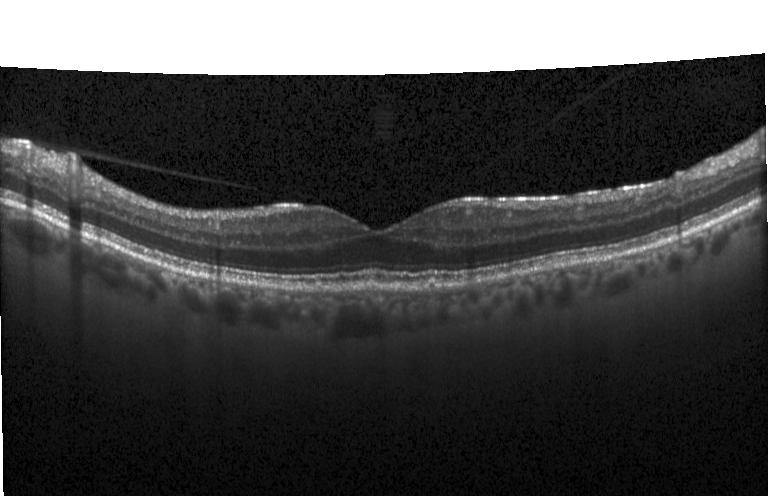

Spectral-domain optical coherence tomography; Heidelberg Spectralis; fovea-centered; optical coherence tomography scan.
Finding: sub-RPE drusenoid deposits.